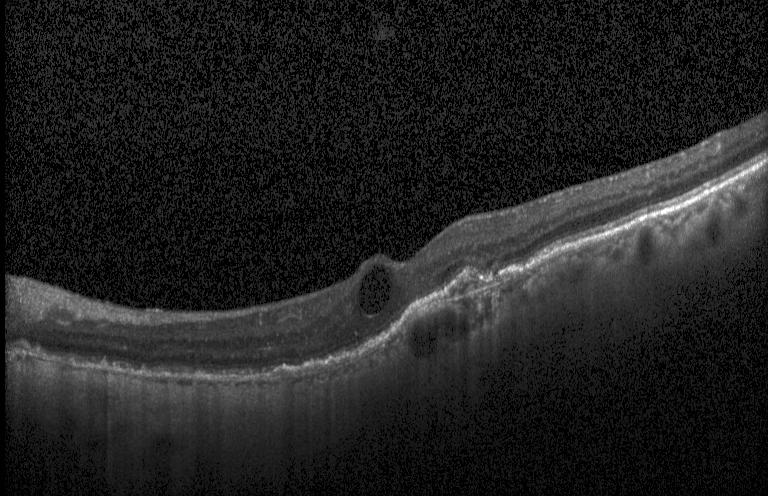 Dx: CNV.